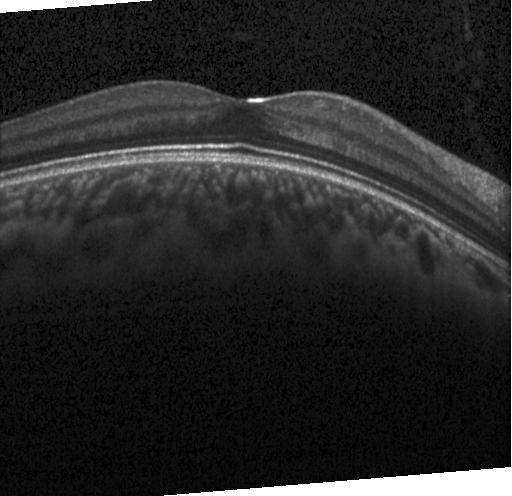 Heidelberg Spectralis OCT system; OCT line scan; spectral-domain OCT
Diagnosis: neither choroidal neovascularization, diabetic macular edema, nor drusen.